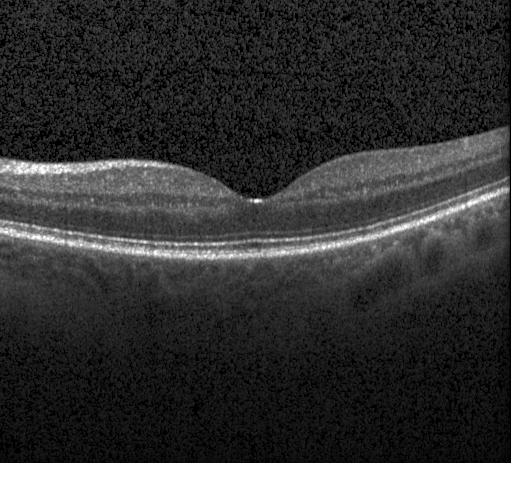

Impression: no choroidal neovascularization, diabetic macular edema, or drusen.